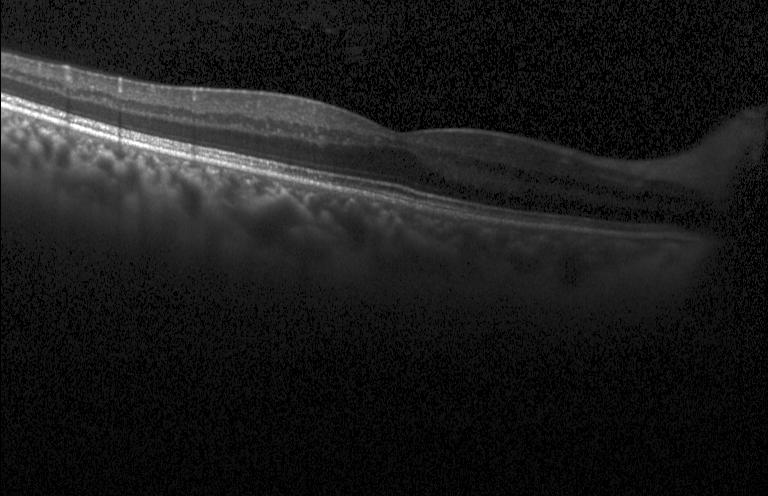

Dx: no CNV, DME, or drusen.